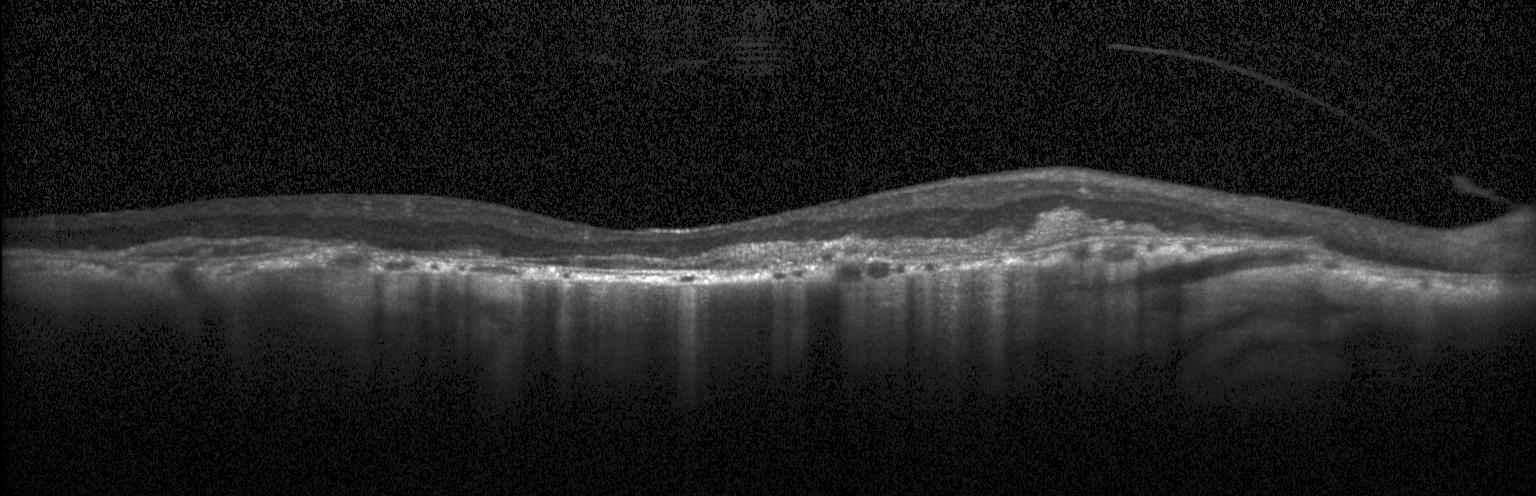

OCT line scan. Assessment: choroidal neovascularization (CNV).